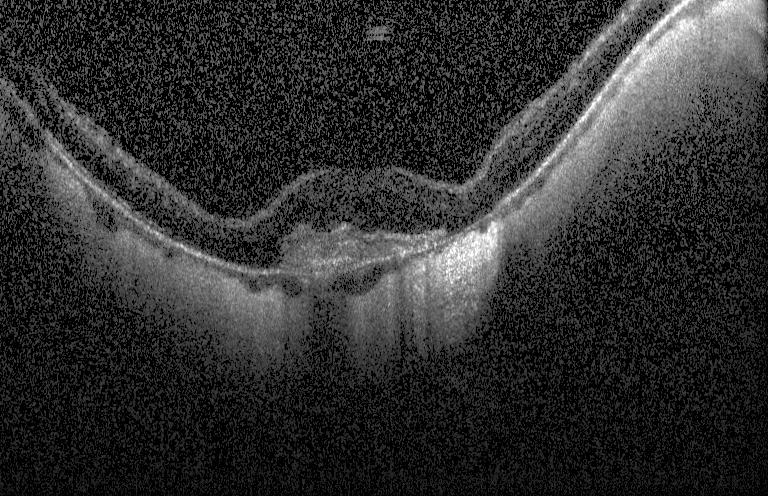 Instrument: Heidelberg Spectralis. Optical coherence tomography B-scan. Centered on the fovea. Spectral-domain OCT
Diagnosis: choroidal neovascularization (CNV).